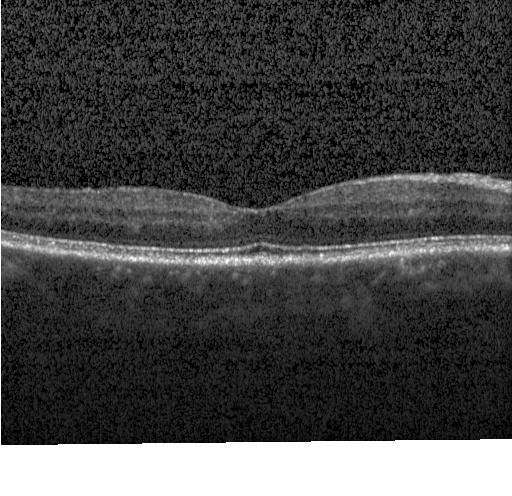

OCT scan showing no choroidal neovascularization, diabetic macular edema, or drusen.